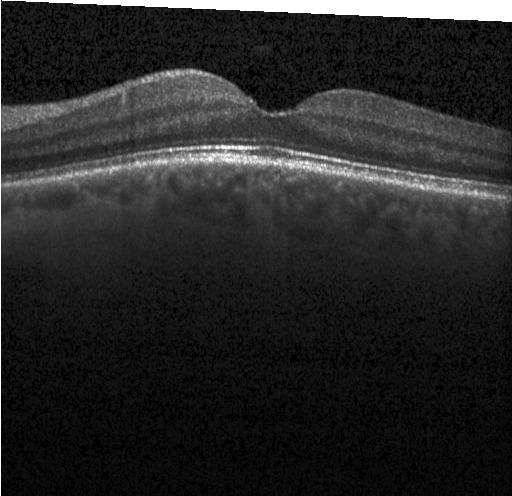

Spectral-domain optical coherence tomography; through the macula; instrument: Heidelberg Spectralis; OCT line scan. Diagnosis: no evidence of choroidal neovascularization, diabetic macular edema, or drusen.